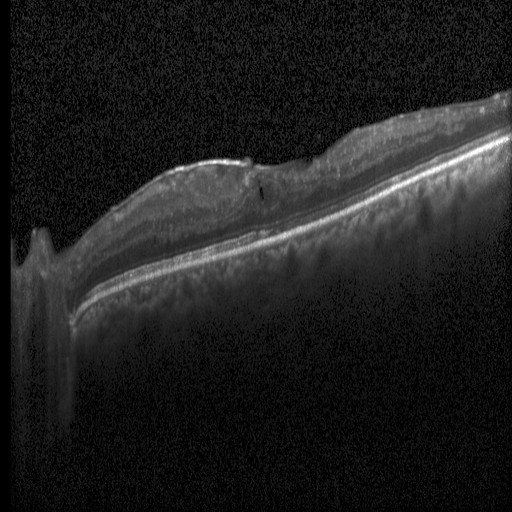 Macular scan. Spectral-domain OCT. Instrument: Heidelberg Spectralis. Retinal OCT cross-section
Impression: DME.